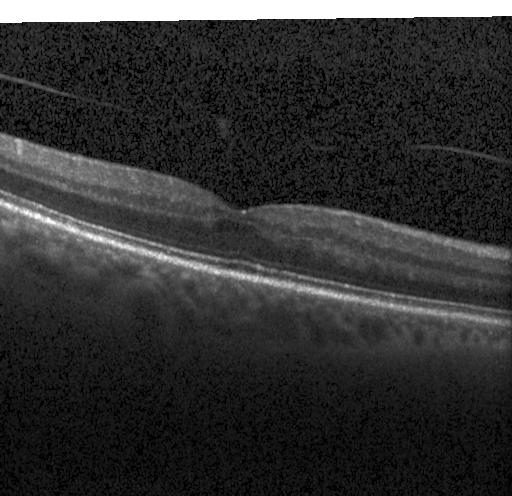
Finding: neither choroidal neovascularization, diabetic macular edema, nor drusen.